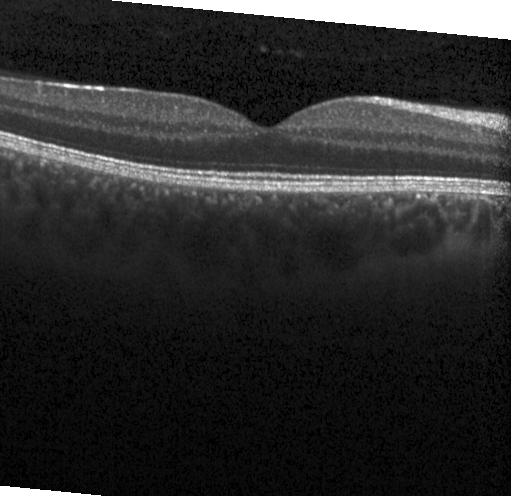
Finding: no evidence of CNV, DME, or drusen.